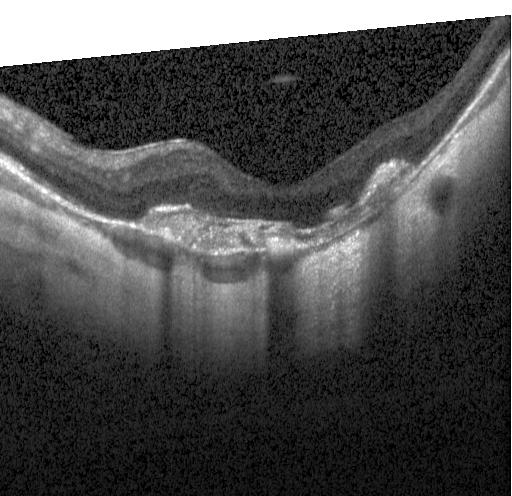

Diagnosis: choroidal neovascularization.